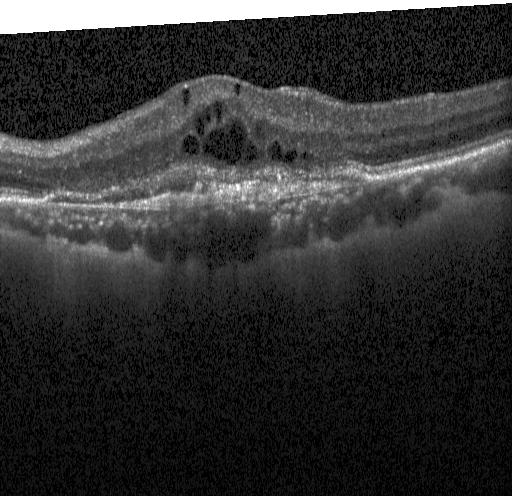
Retinal OCT B-scan · horizontal scan through the fovea · SD-OCT · Heidelberg Spectralis — Assessment: a choroidal neovascular membrane.